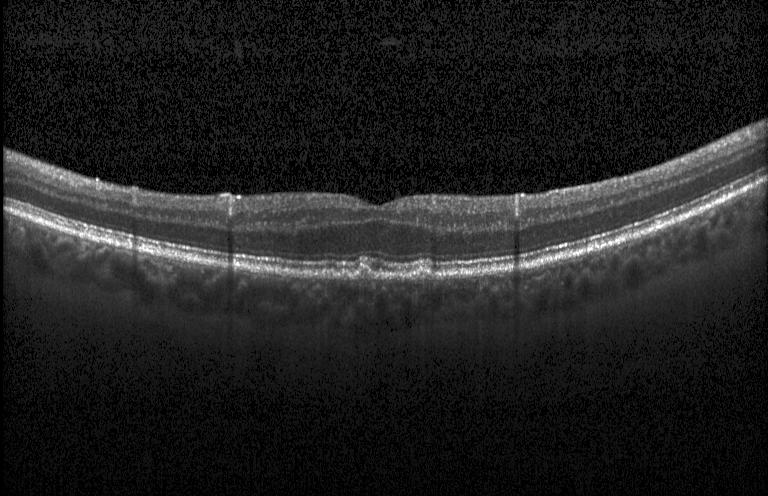

Finding: multiple drusen.